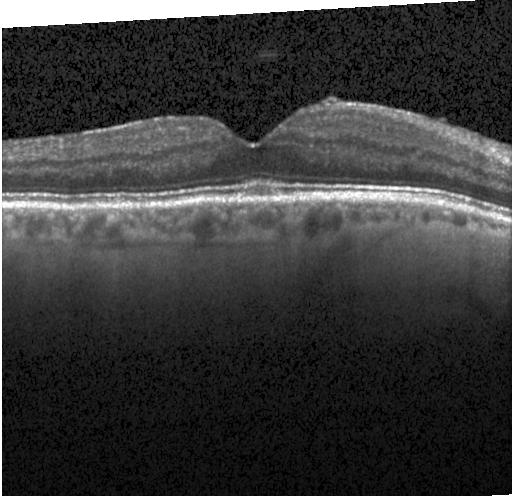 Through the macula, SD-OCT, OCT B-scan
Dx: no choroidal neovascularization, diabetic macular edema, or drusen.